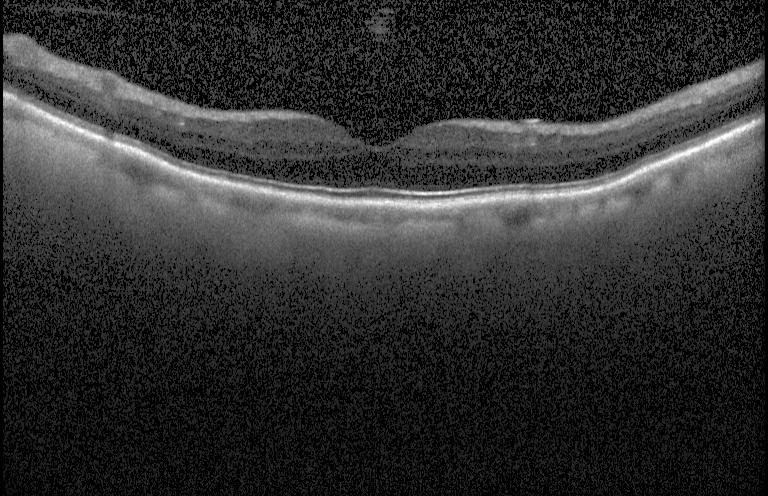

Retinal OCT cross-section. Diagnosis: neither choroidal neovascularization, diabetic macular edema, nor drusen.